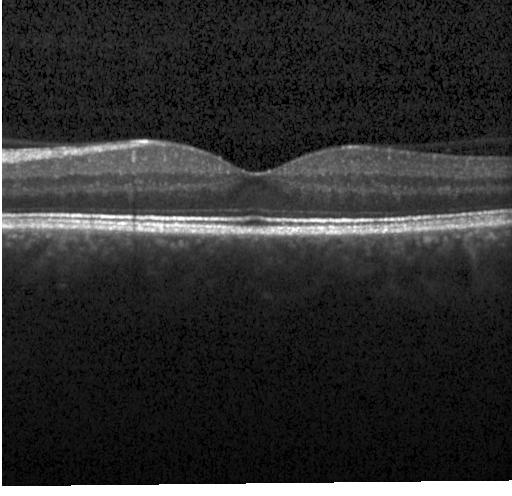 Retinal OCT cross-section · horizontal scan through the fovea · Heidelberg Spectralis OCT system · spectral-domain OCT — The scan shows no choroidal neovascularization, no diabetic macular edema, and no drusen.